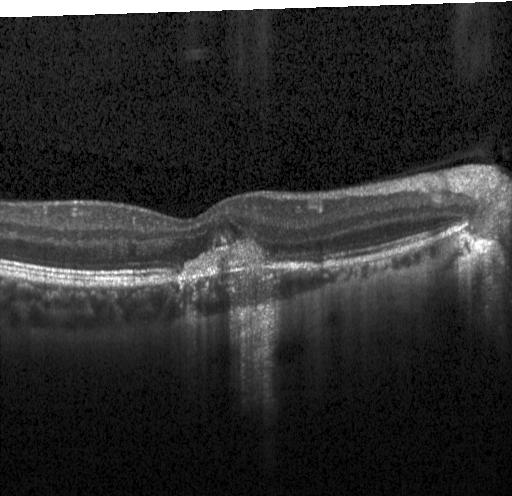 Dx: CNV.